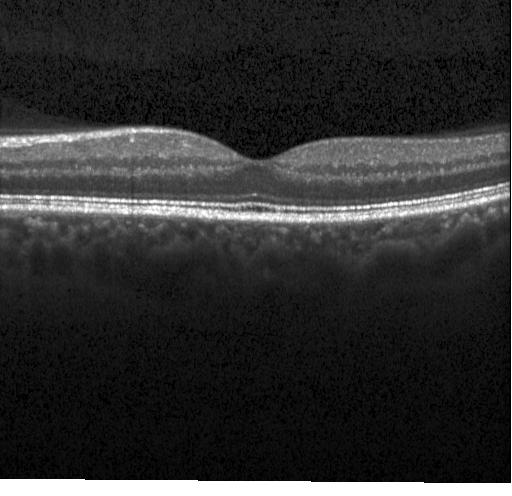 Finding: neither CNV, DME, nor drusen.